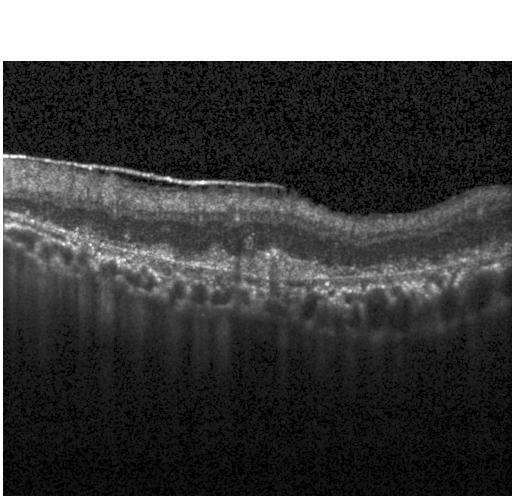
Spectral-domain OCT B-scan: choroidal neovascularization (CNV).